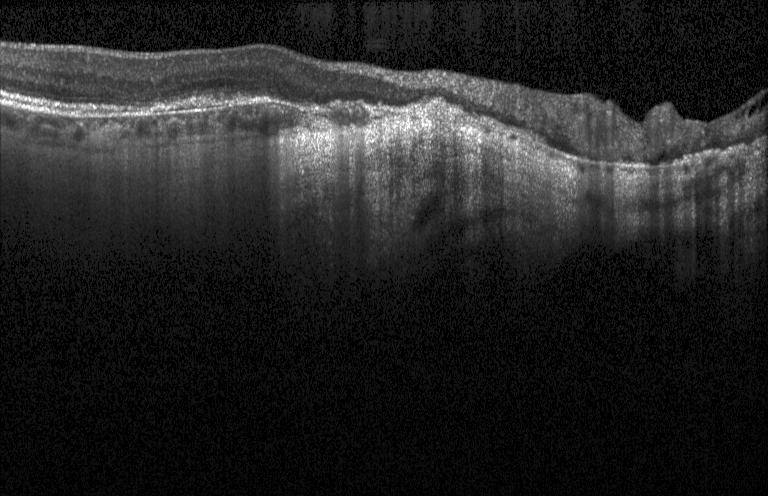 Dx: choroidal neovascularization.